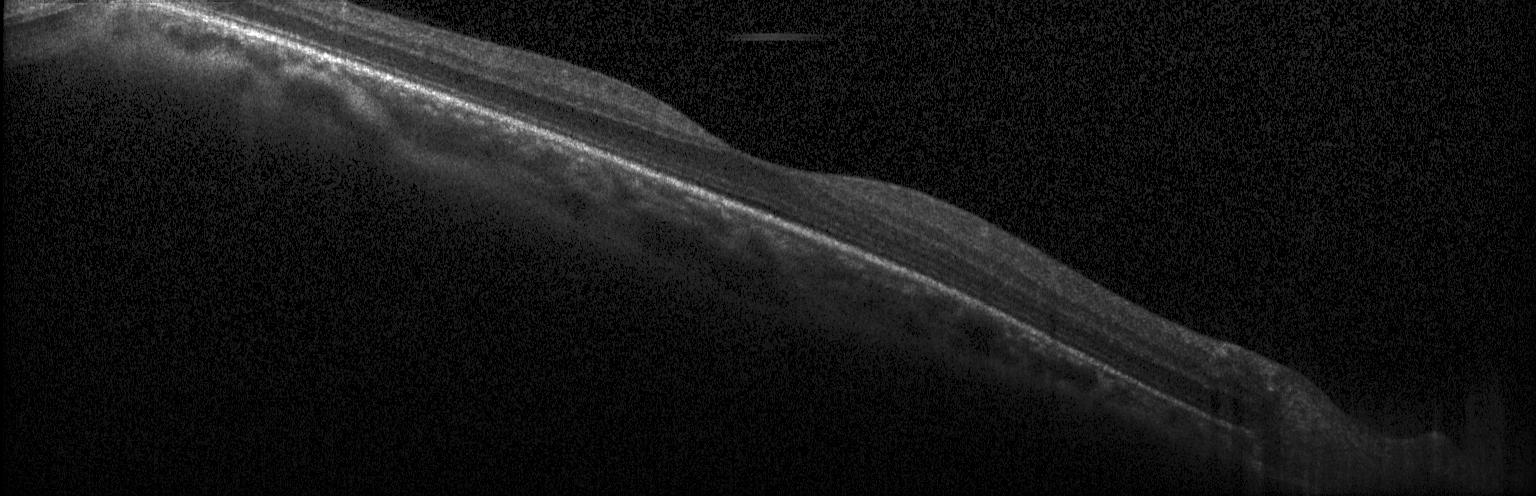
OCT line scan.
Finding: no choroidal neovascularization, no diabetic macular edema, and no drusen.